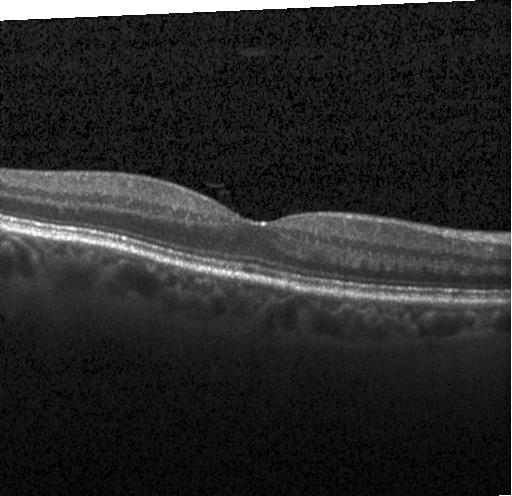

Heidelberg Spectralis OCT system. Retinal OCT B-scan
Neither CNV, DME, nor drusen.